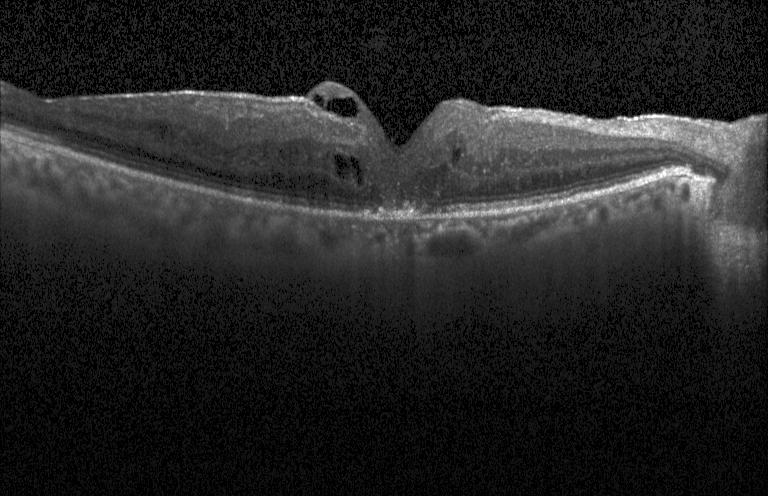 OCT B-scan · spectral-domain optical coherence tomography · Heidelberg Spectralis.
Impression: diabetic macular edema.